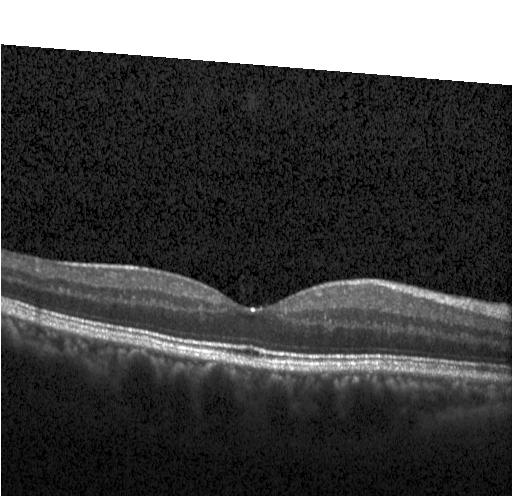
Retinal OCT cross-section showing no choroidal neovascularization, diabetic macular edema, or drusen.